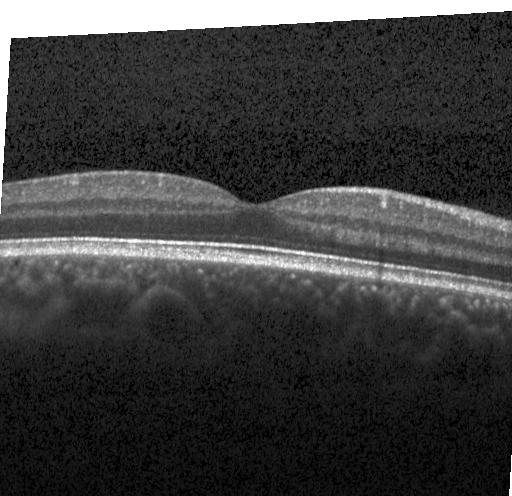
OCT line scan, spectral-domain OCT, through the macula. Dx: no choroidal neovascularization, no diabetic macular edema, and no drusen.